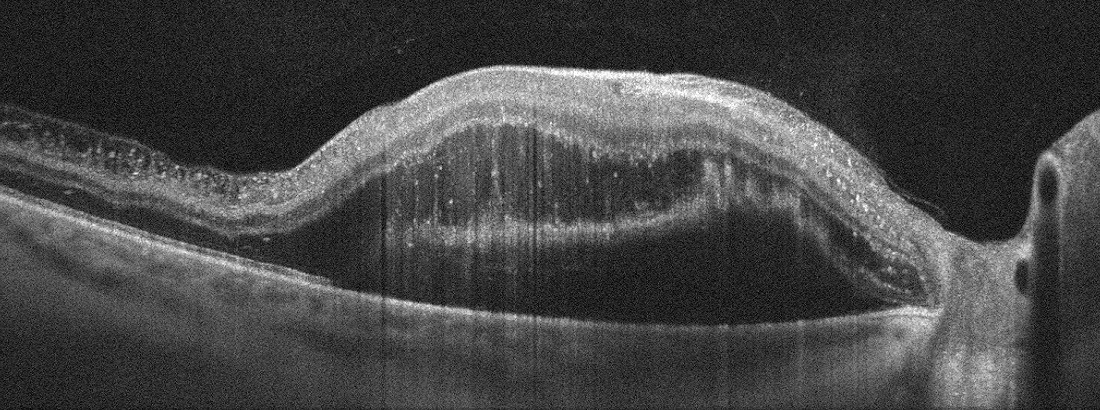
Retinal OCT B-scan, macular scan.
This B-scan demonstrates retinal vein occlusion (RVO).